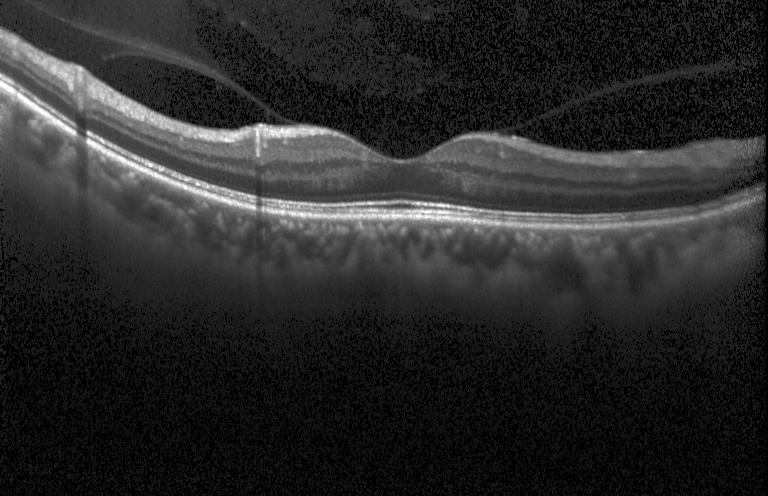
Macular OCT demonstrating no choroidal neovascularization, diabetic macular edema, or drusen.